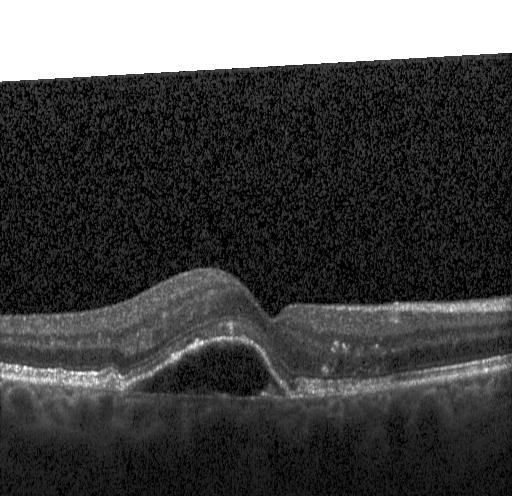
OCT finding: a choroidal neovascular membrane.